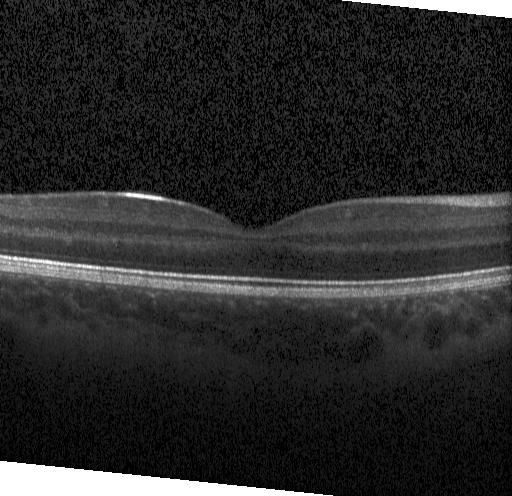 Diagnosis: no evidence of CNV, DME, or drusen.